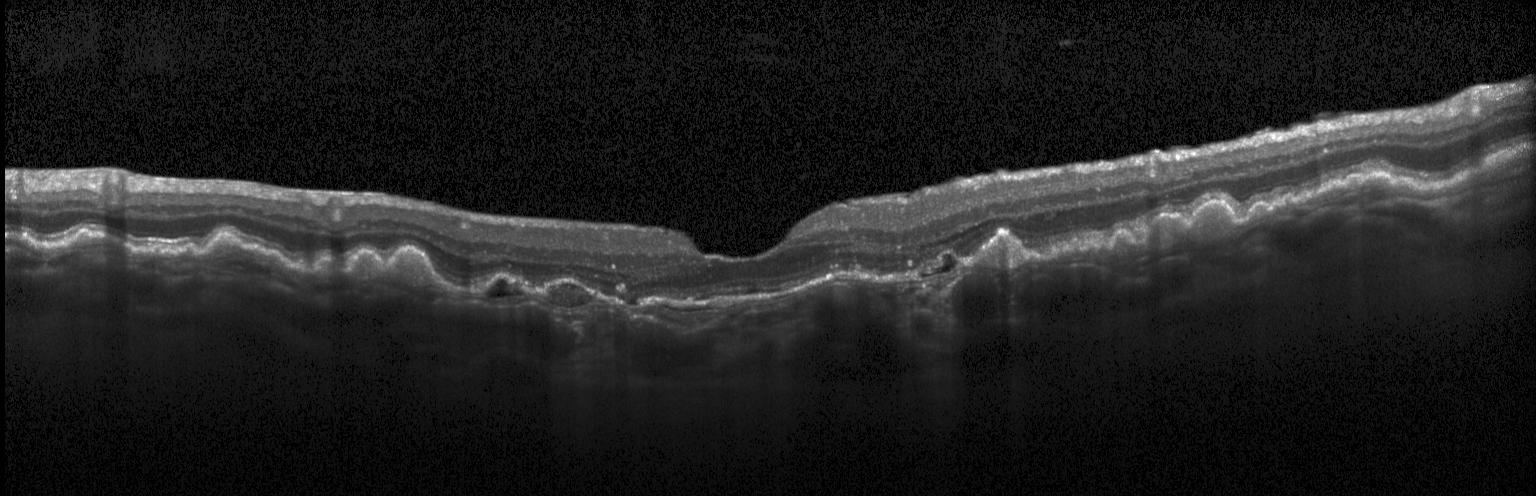

Impression: a choroidal neovascular membrane.